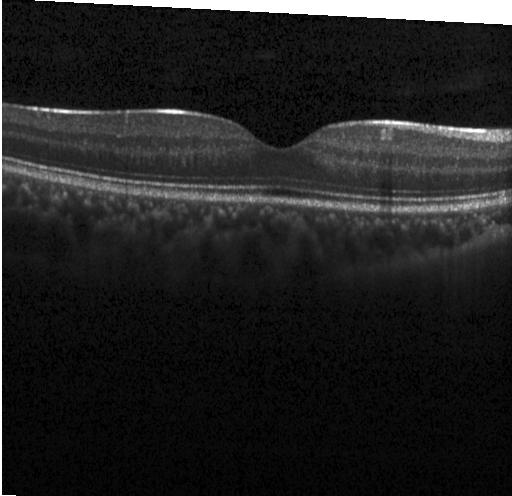 Finding: neither choroidal neovascularization, diabetic macular edema, nor drusen.